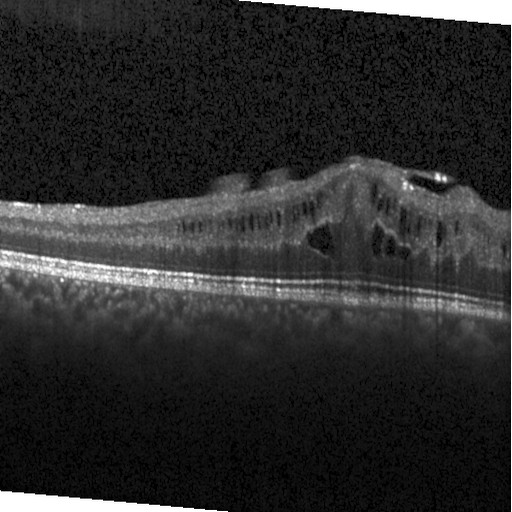
Retinal OCT cross-section · spectral-domain OCT · Heidelberg Spectralis — Assessment: DME.